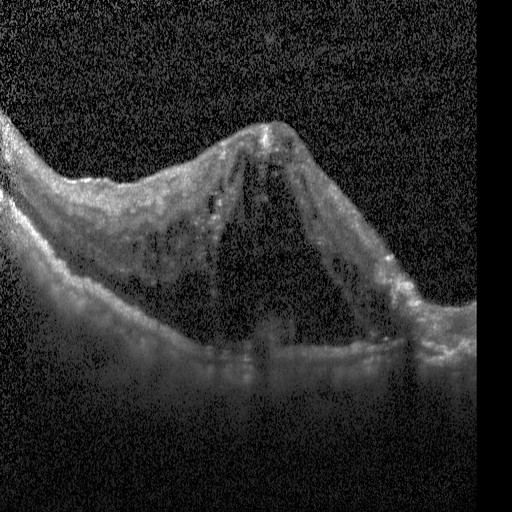
Retinal OCT cross-section
Finding: DME.